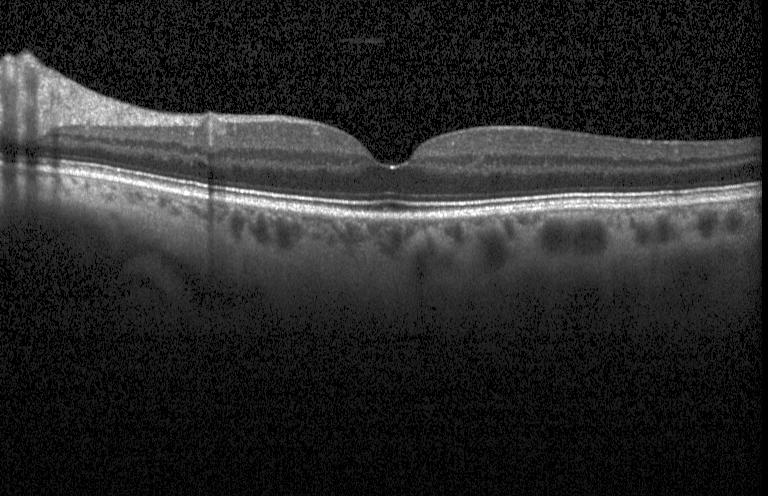
Macular scan. Spectral-domain OCT. Optical coherence tomography scan
Finding: no choroidal neovascularization, diabetic macular edema, or drusen.